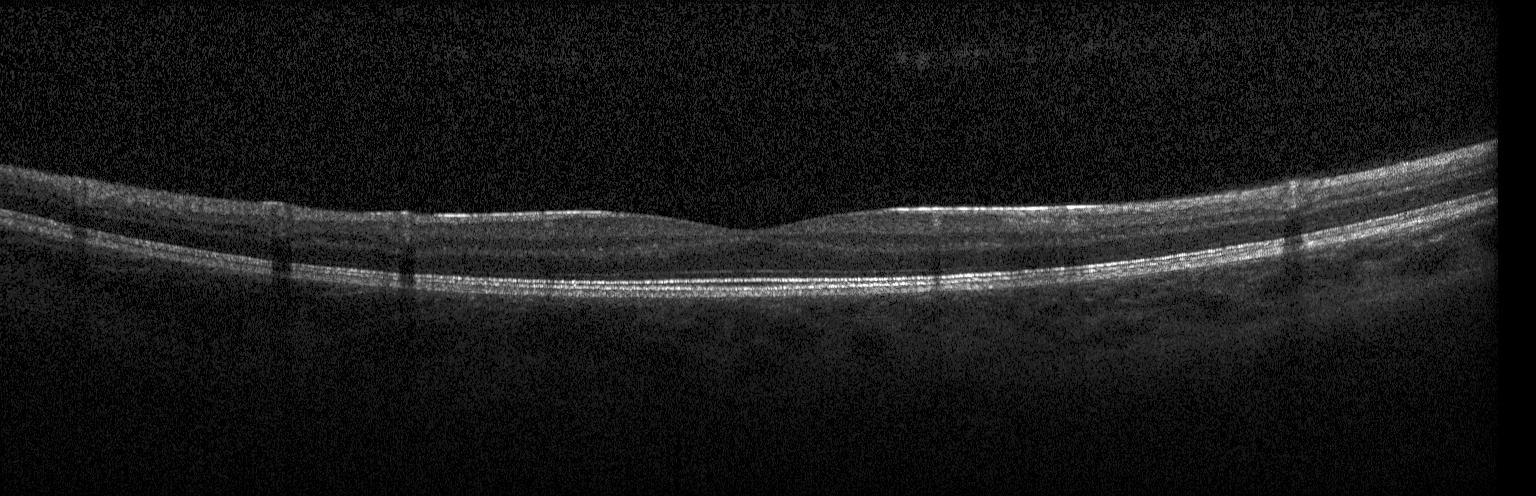 This B-scan demonstrates no CNV, no DME, and no drusen.